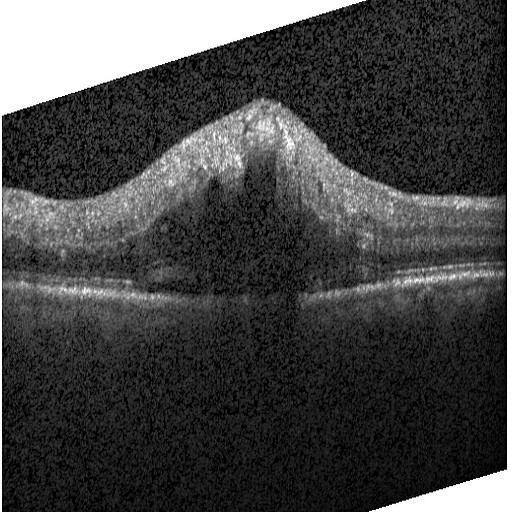

Diagnosis: diabetic macular edema (DME).